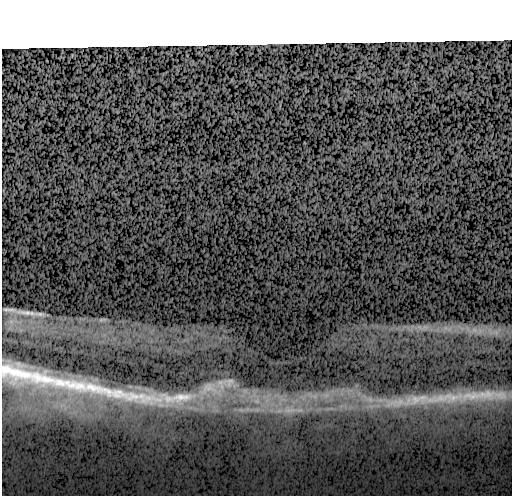 Through the macula. Retinal OCT B-scan — The scan shows choroidal neovascularization (CNV).